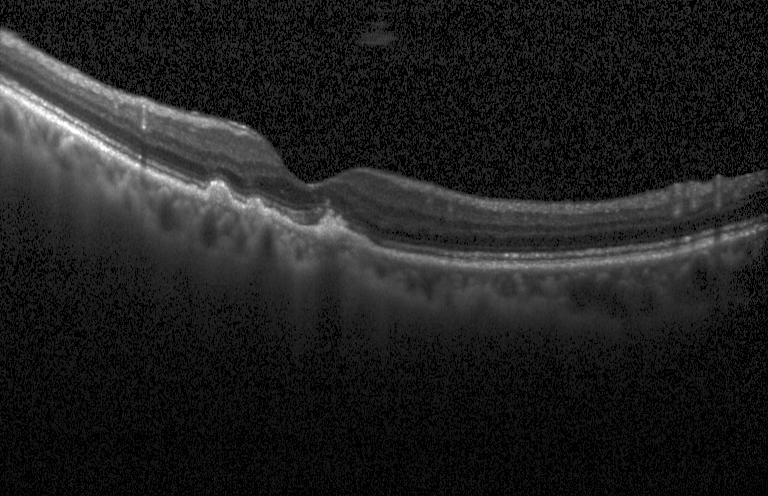 Retinal OCT cross-section. SD-OCT. Macular scan.
Finding: a choroidal neovascular membrane.